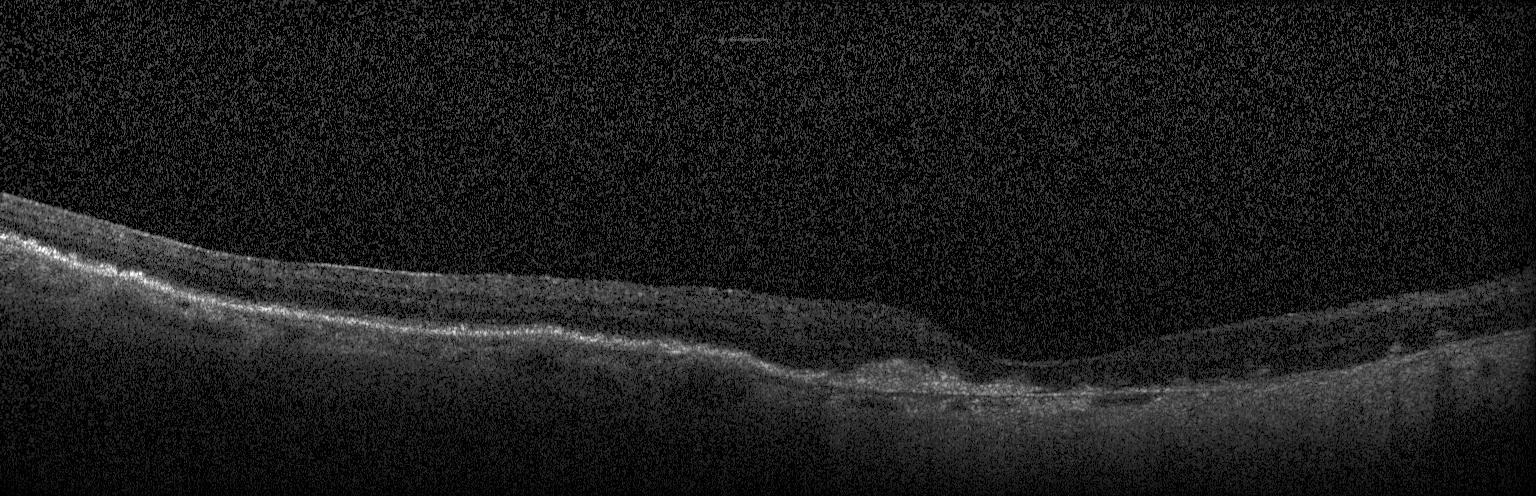
Diagnosis: choroidal neovascularization.